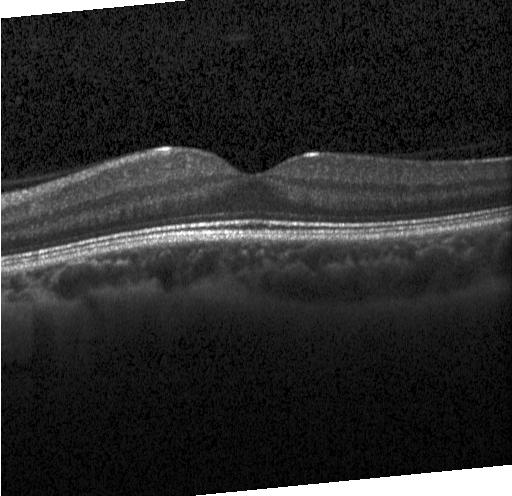 Heidelberg Spectralis · OCT line scan · spectral-domain OCT · centered on the fovea — Diagnosis: no CNV, DME, or drusen.